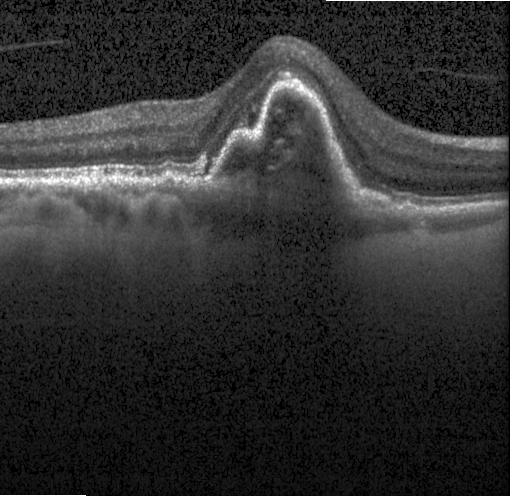
Finding: choroidal neovascularization.